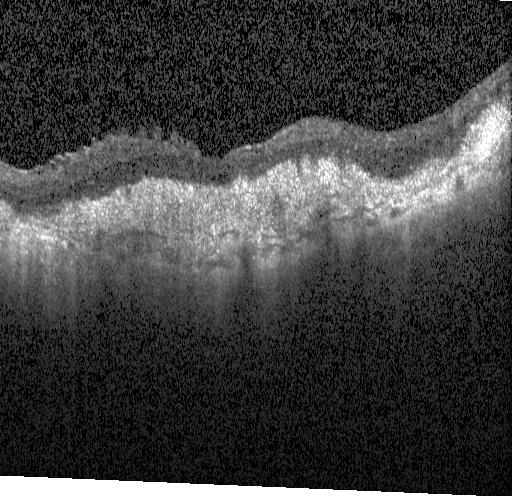

Optical coherence tomography B-scan — OCT finding: a choroidal neovascular membrane.